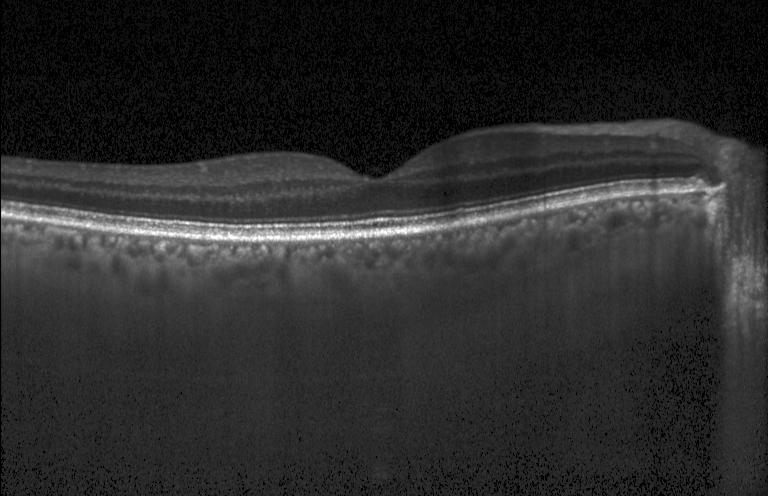

Optical coherence tomography scan, macular scan
Dx: no evidence of choroidal neovascularization, diabetic macular edema, or drusen.